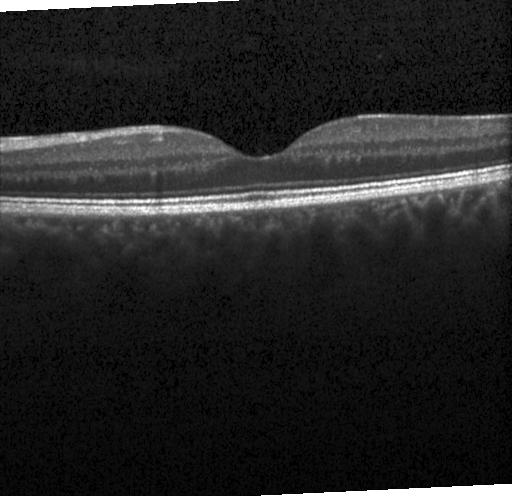

Retinal OCT cross-section. OCT finding: neither CNV, DME, nor drusen.